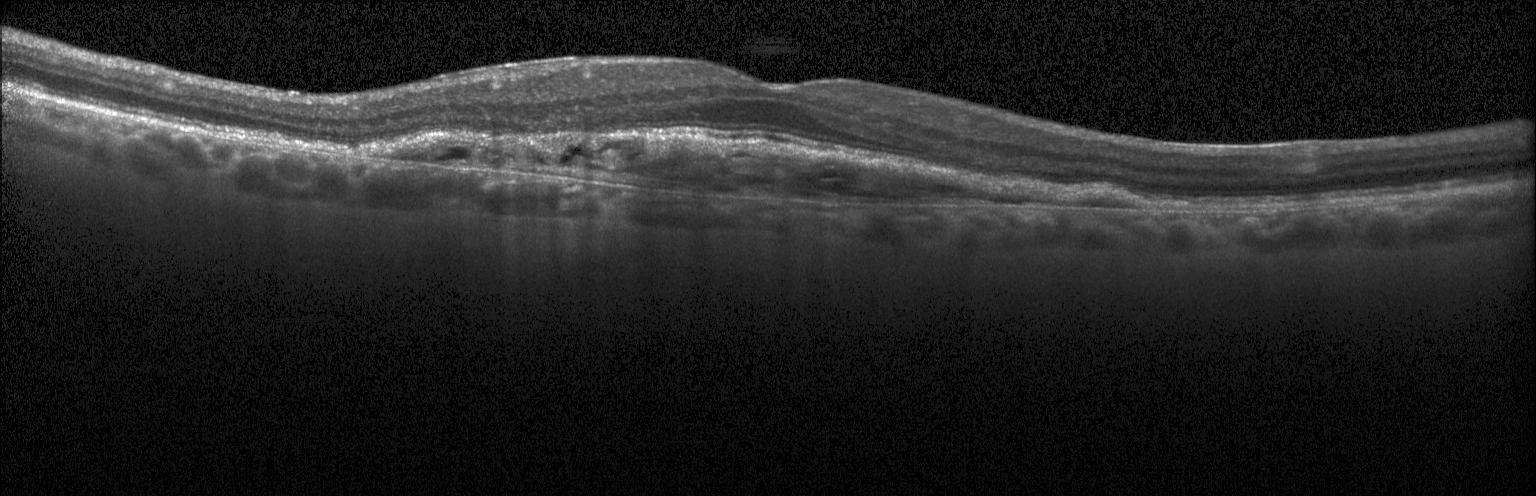
Retinal OCT B-scan. SD-OCT.
Choroidal neovascularization.